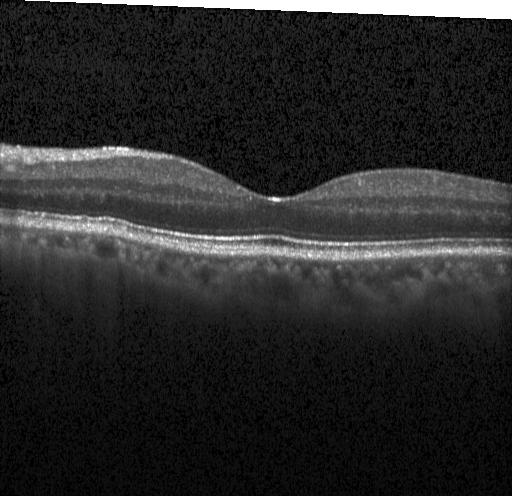

Dx: no evidence of choroidal neovascularization, diabetic macular edema, or drusen.